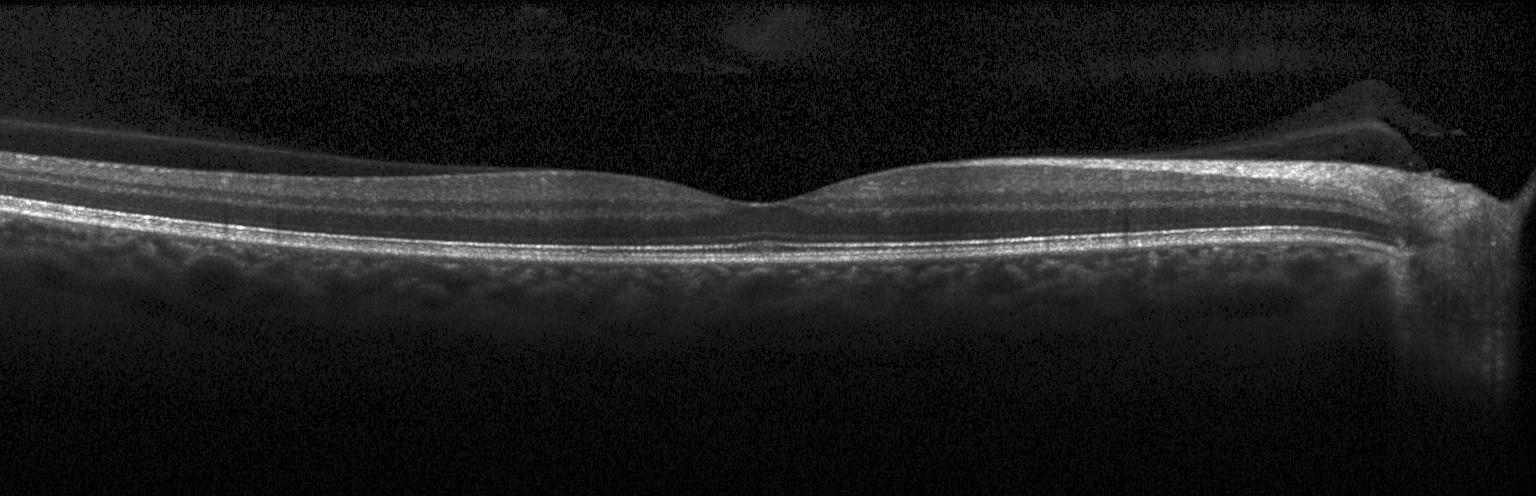 Instrument: Heidelberg Spectralis; optical coherence tomography scan; fovea-centered; spectral-domain optical coherence tomography — Dx: no choroidal neovascularization, no diabetic macular edema, and no drusen.